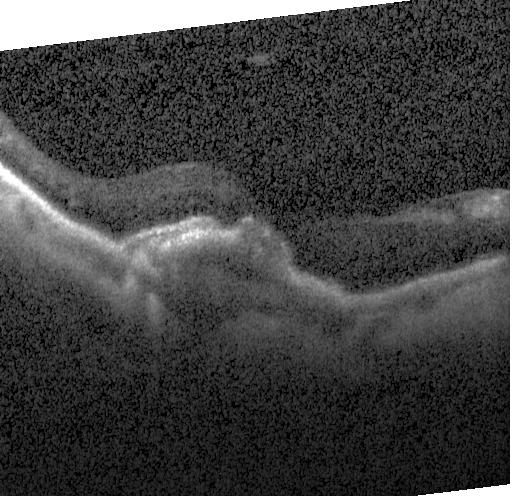

OCT B-scan — Diagnosis: CNV.